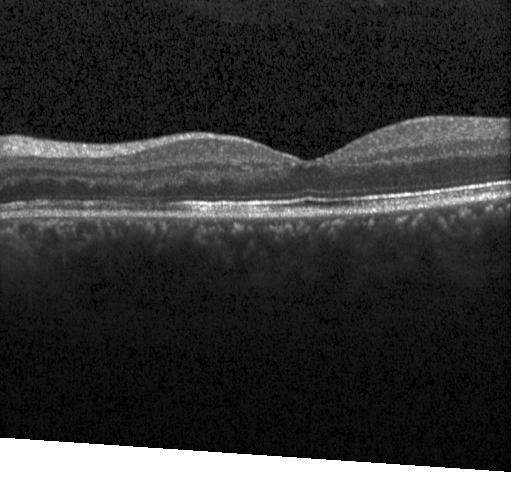
Retinal OCT B-scan. Finding: no CNV, no DME, and no drusen.